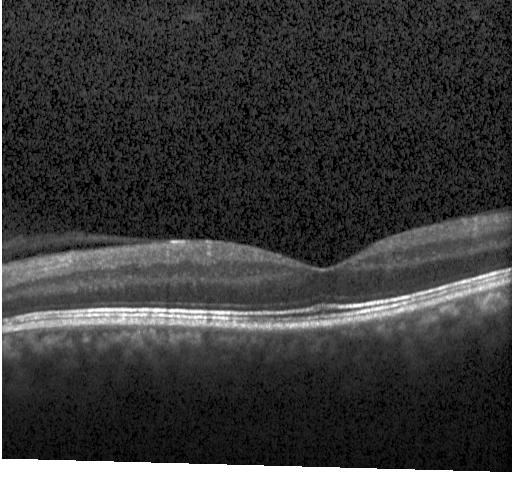
This B-scan demonstrates no CNV, DME, or drusen.